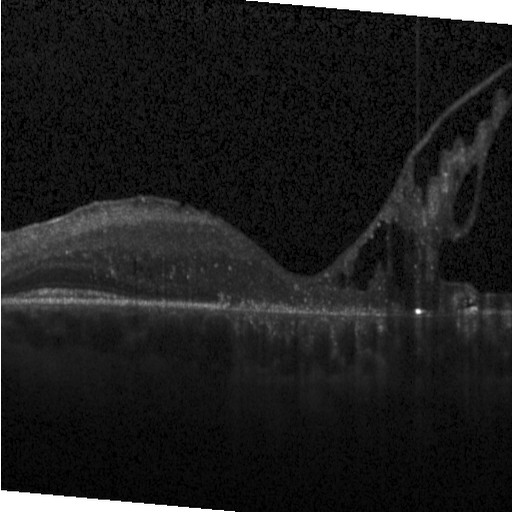
OCT B-scan. Macular scan. Assessment: DME.